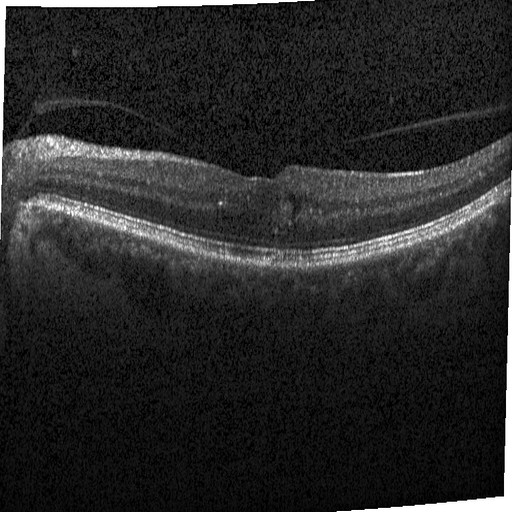

Impression: diabetic macular edema (DME).